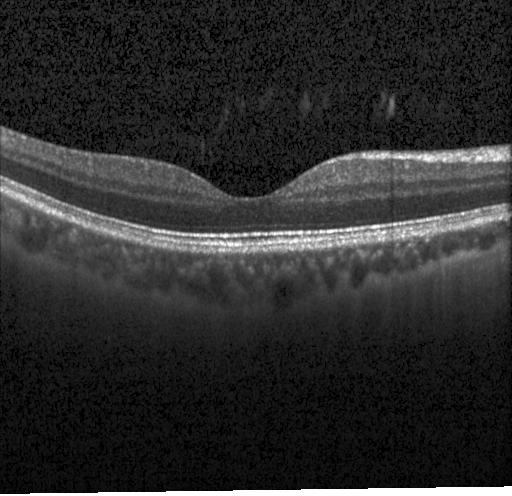 Diagnosis: no choroidal neovascularization, diabetic macular edema, or drusen.